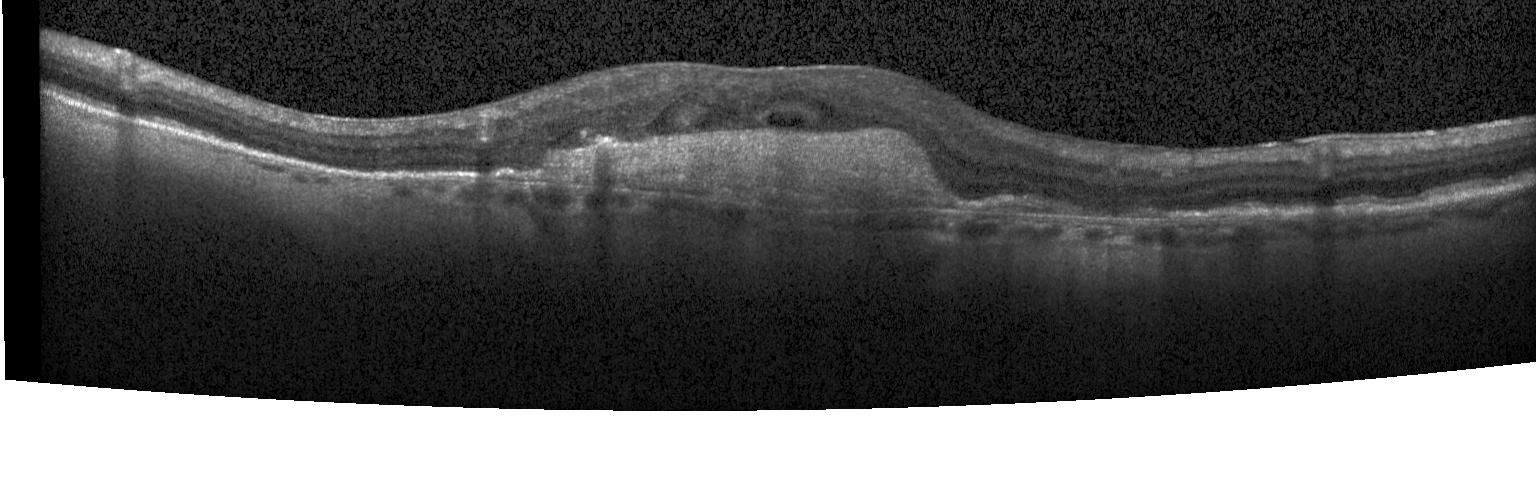
Macular OCT: a choroidal neovascular membrane.